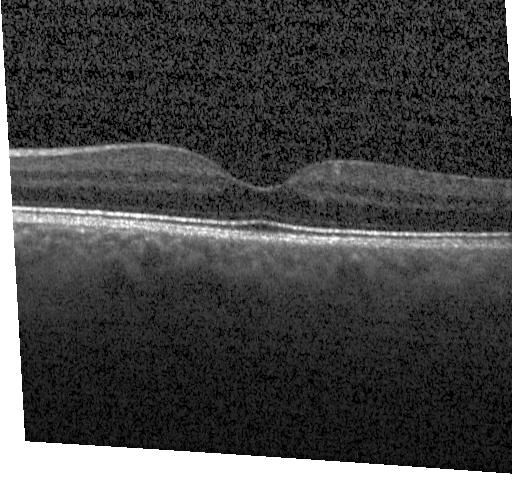

Impression: neither choroidal neovascularization, diabetic macular edema, nor drusen.